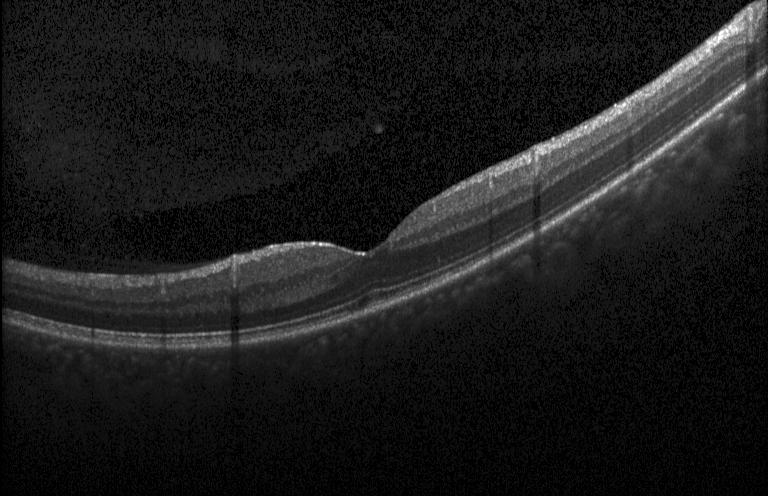
OCT B-scan showing no choroidal neovascularization, no diabetic macular edema, and no drusen.